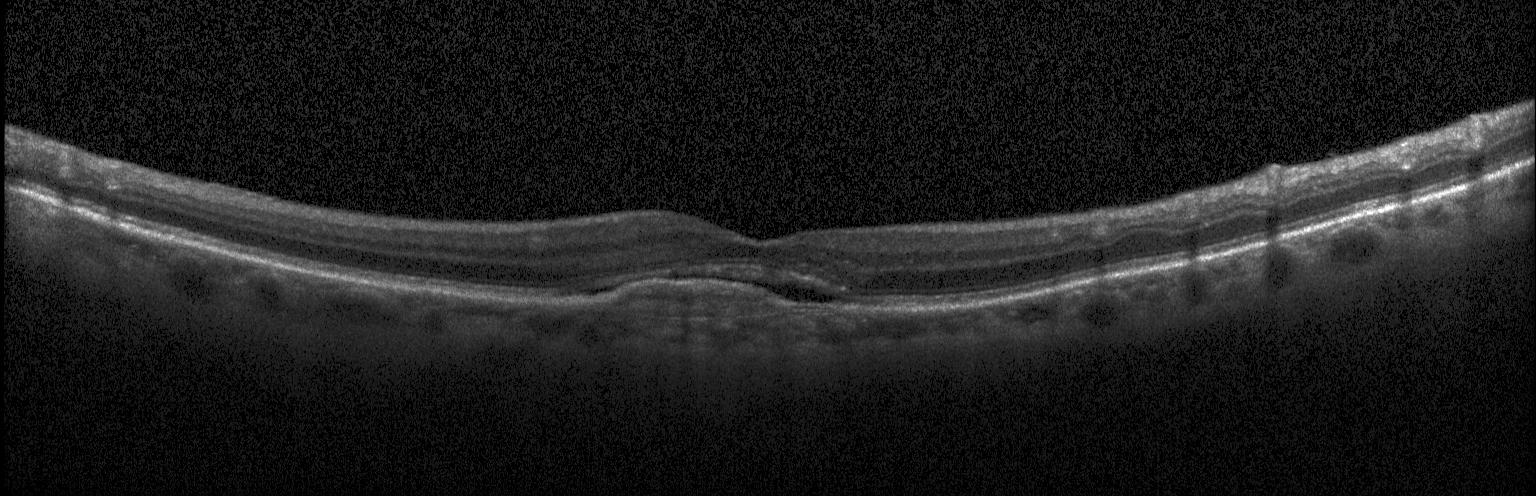
Spectral-domain optical coherence tomography · optical coherence tomography scan · through the macula
A choroidal neovascular membrane.